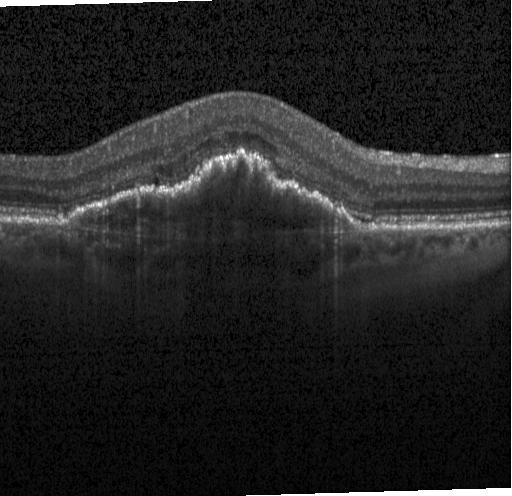

OCT line scan — Dx: a choroidal neovascular membrane.